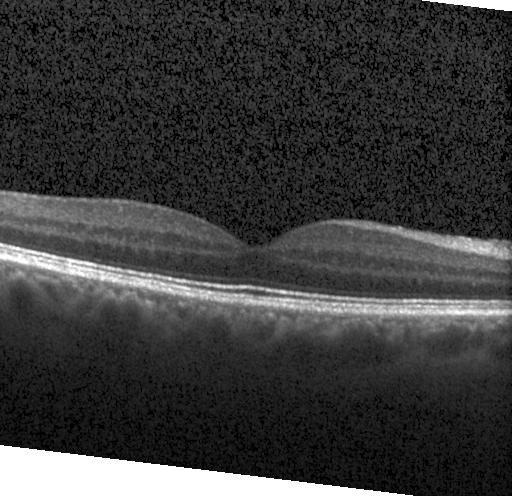
OCT B-scan, acquired on a Heidelberg Spectralis
Macular OCT: no evidence of choroidal neovascularization, diabetic macular edema, or drusen.